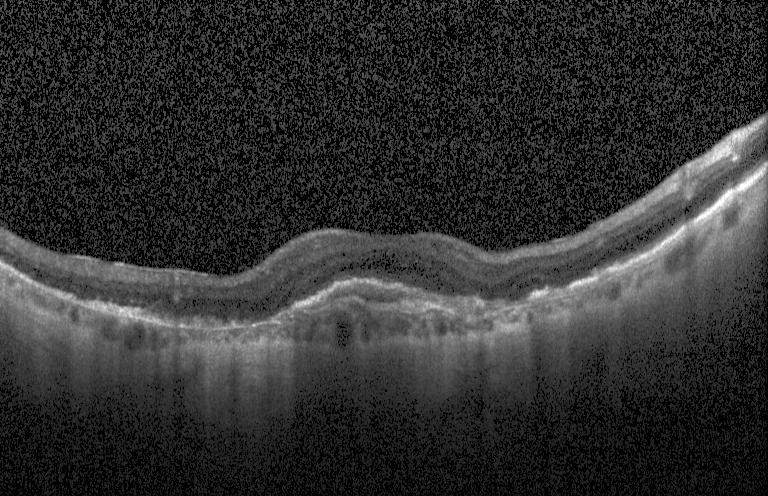 The scan shows a choroidal neovascular membrane.